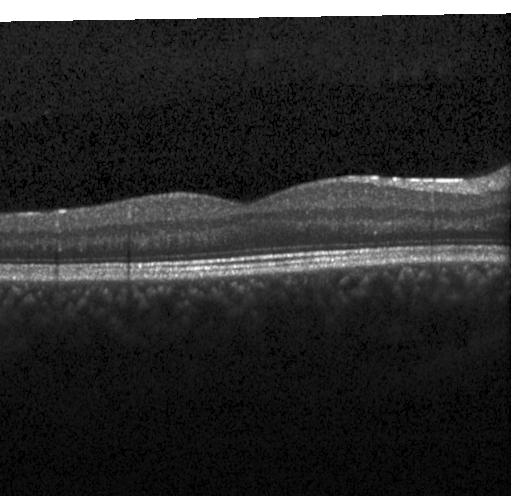

Heidelberg Spectralis, centered on the fovea, optical coherence tomography B-scan, spectral-domain OCT.
Macular OCT: no evidence of choroidal neovascularization, diabetic macular edema, or drusen.